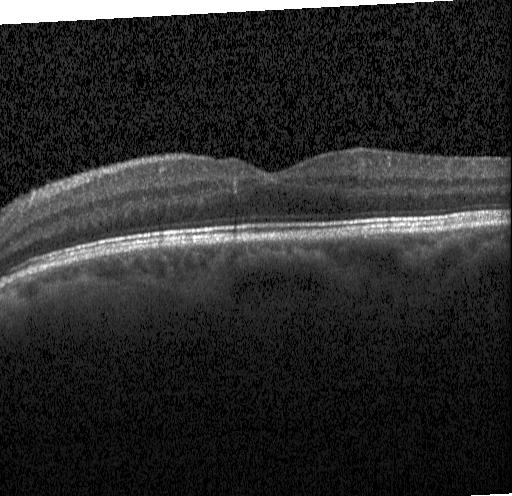
Finding: neither choroidal neovascularization, diabetic macular edema, nor drusen.